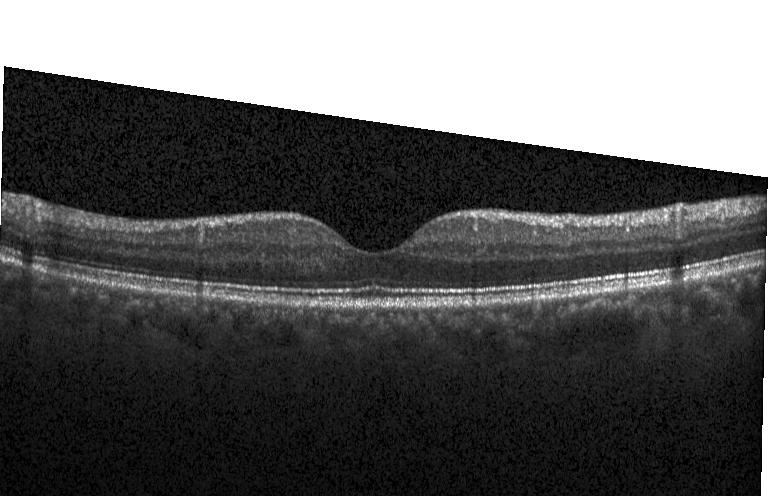 Diagnosis: no choroidal neovascularization, no diabetic macular edema, and no drusen.